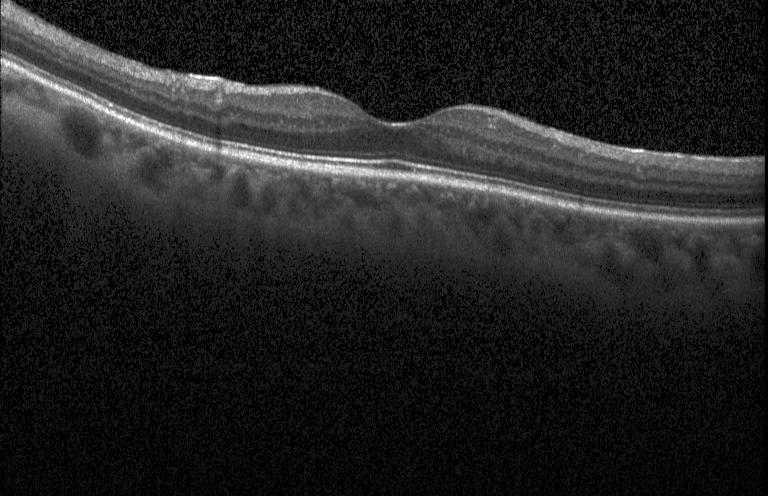

OCT B-scan — Assessment: neither choroidal neovascularization, diabetic macular edema, nor drusen.